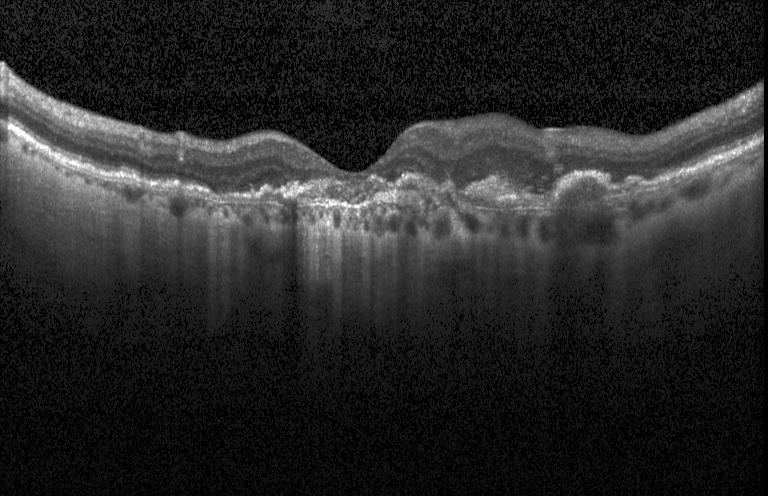

Spectral-domain OCT · retinal OCT cross-section · acquired on a Heidelberg Spectralis — OCT finding: choroidal neovascularization (CNV).